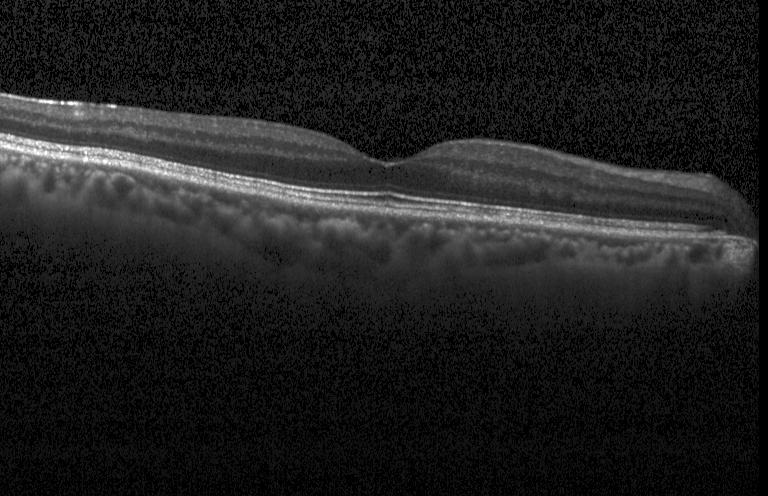

This B-scan demonstrates no choroidal neovascularization, diabetic macular edema, or drusen.